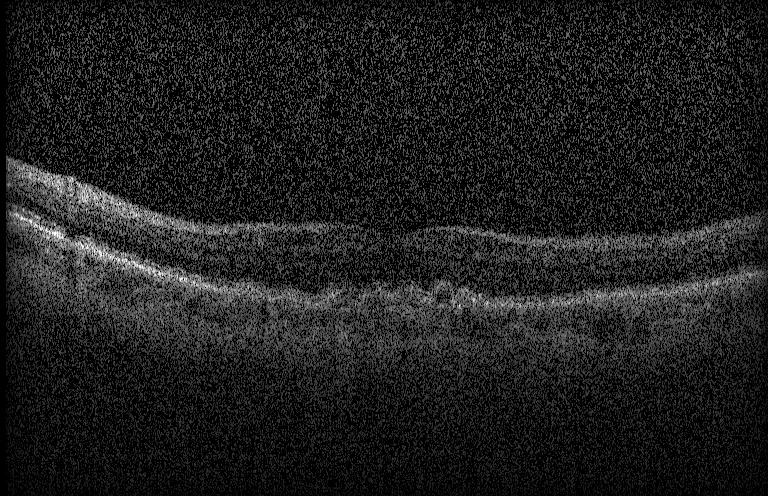

Impression: CNV.